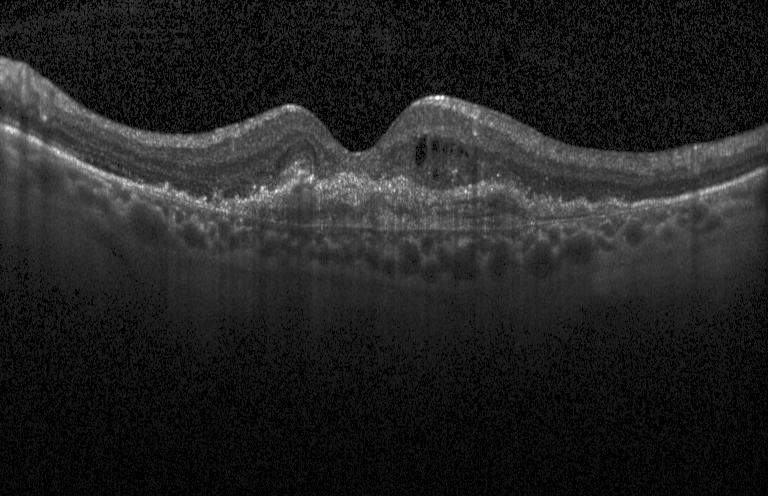 Impression: a choroidal neovascular membrane.